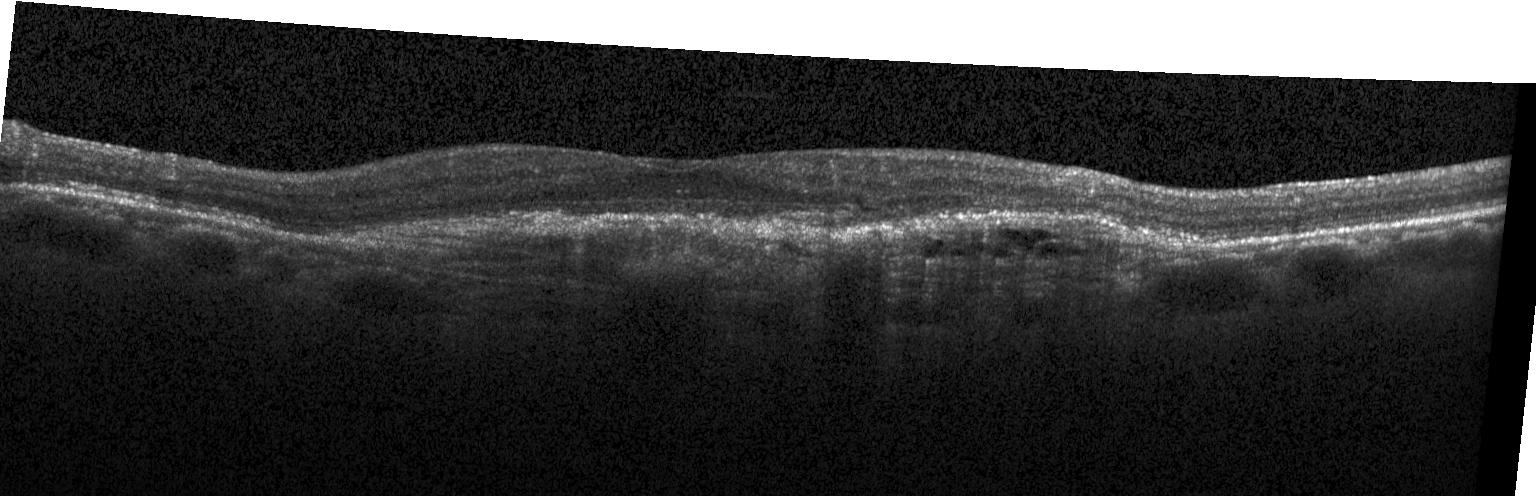 This B-scan demonstrates choroidal neovascularization.